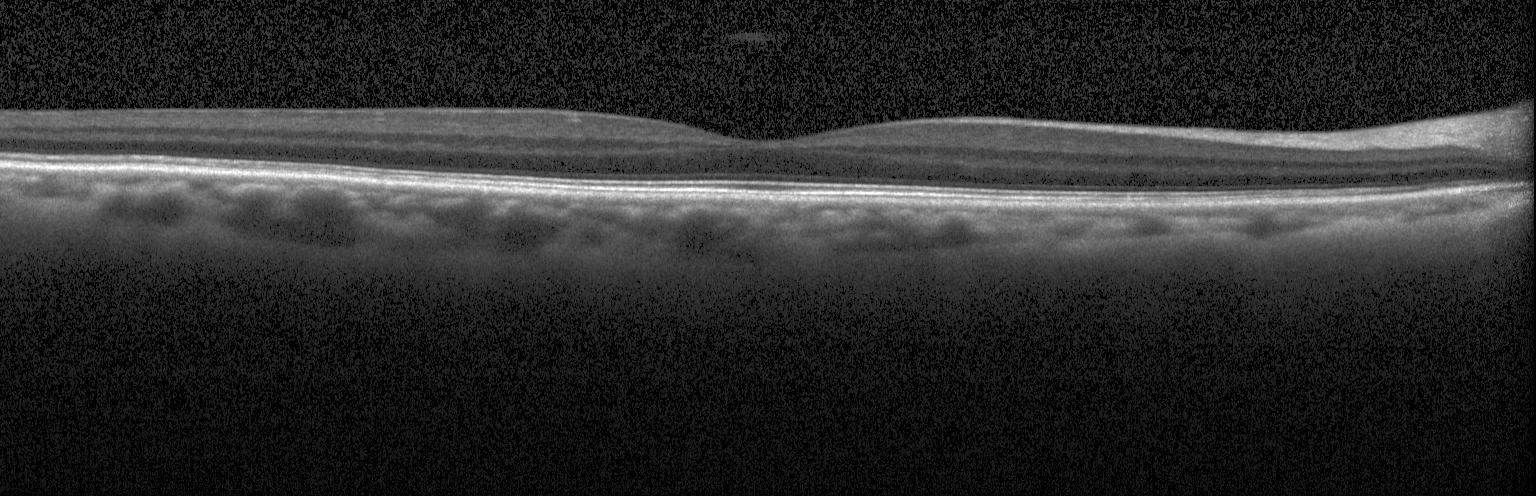
OCT line scan — Dx: no evidence of CNV, DME, or drusen.